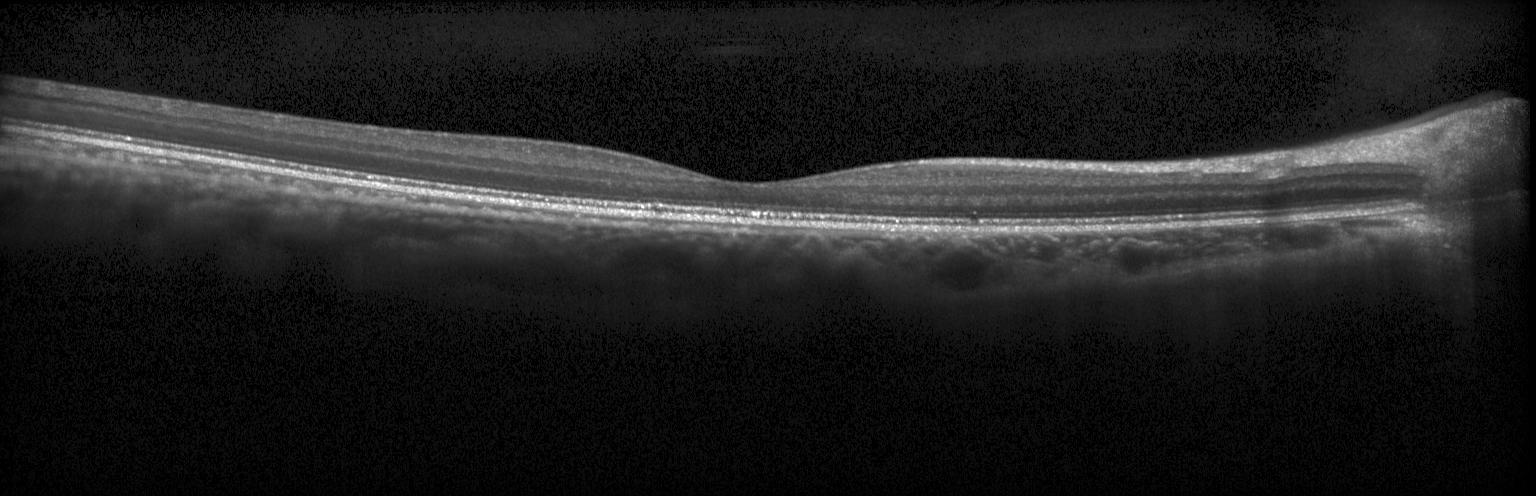
Dx: no CNV, DME, or drusen.